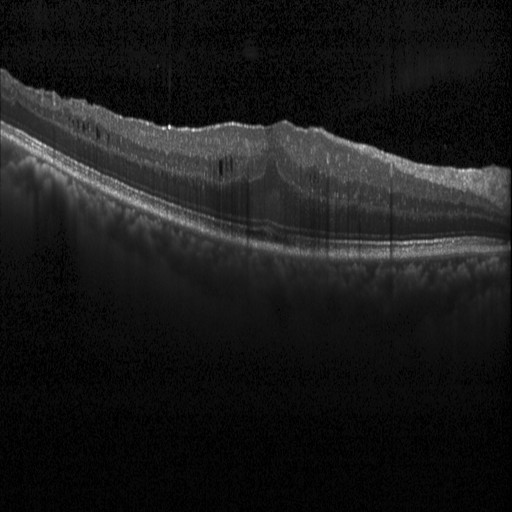

Optical coherence tomography B-scan. Heidelberg Spectralis OCT system. Spectral-domain OCT. Through the macula.
The scan shows DME.